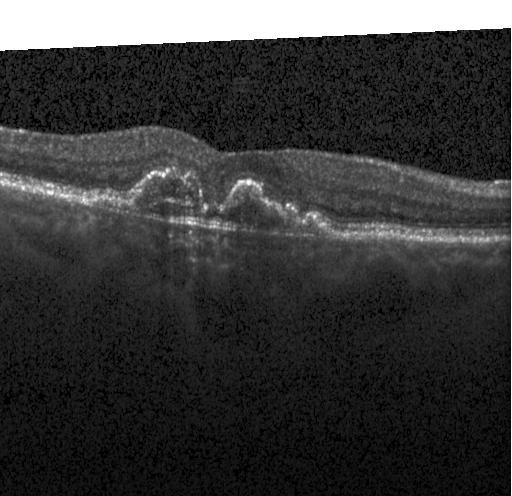
Retinal OCT cross-section
This B-scan demonstrates a choroidal neovascular membrane.